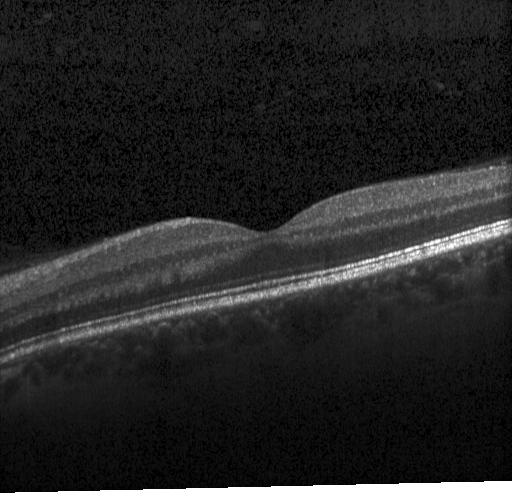
Optical coherence tomography B-scan
The scan shows no evidence of CNV, DME, or drusen.